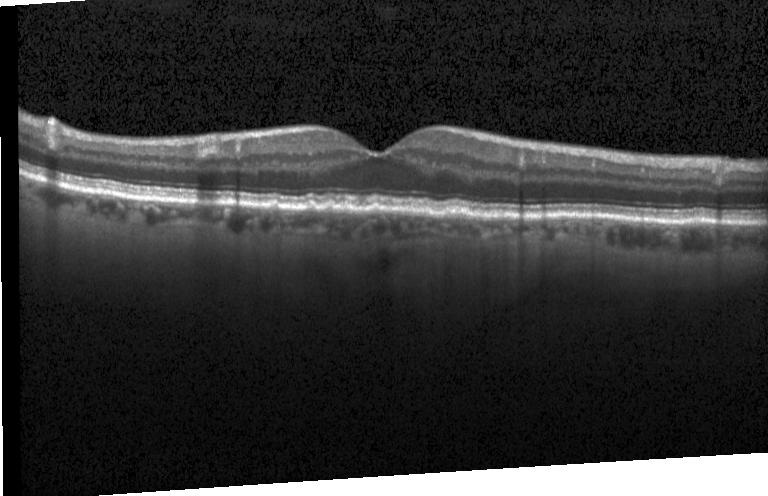
Optical coherence tomography scan
Assessment: multiple drusen.